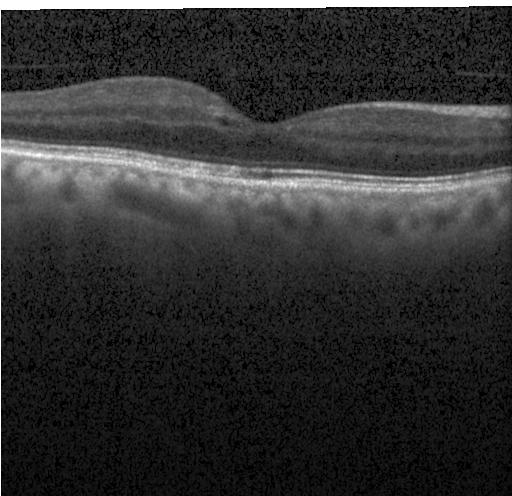

Retinal OCT cross-section — This B-scan demonstrates no CNV, DME, or drusen.